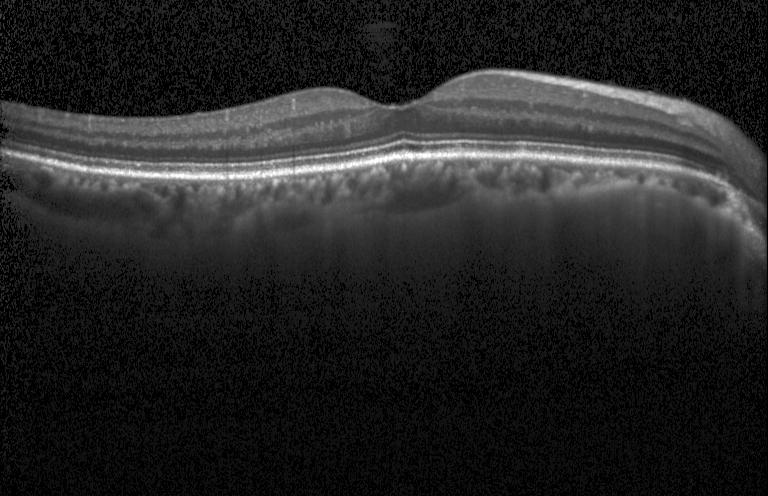
Diagnosis: no choroidal neovascularization, diabetic macular edema, or drusen.